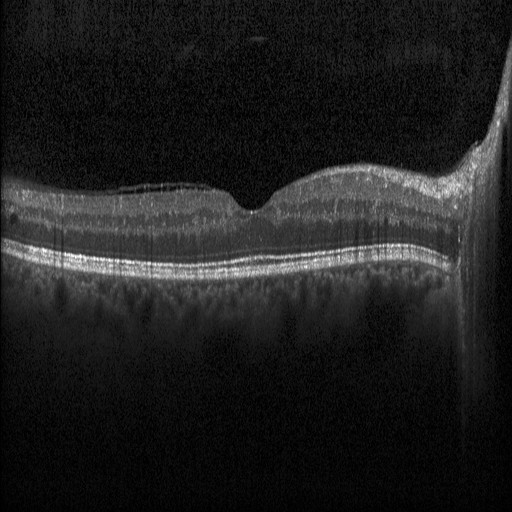 Retinal OCT cross-section, spectral-domain OCT, centered on the fovea.
Finding: diabetic macular edema (DME).